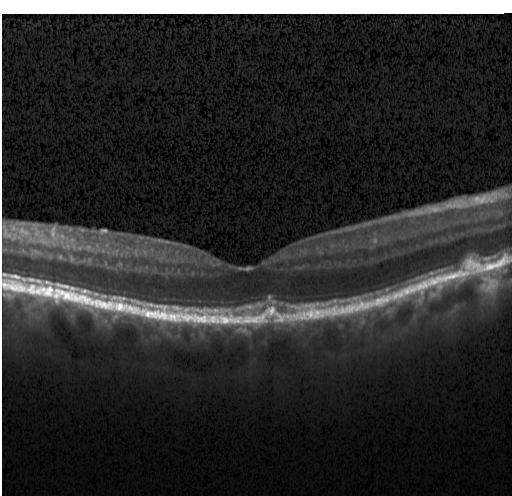
Retinal OCT cross-section showing sub-RPE drusenoid deposits.